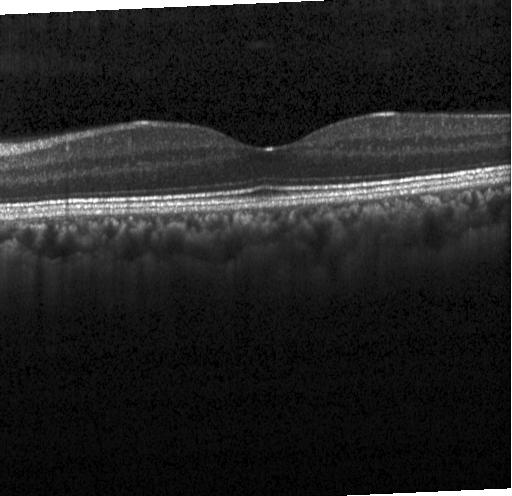
Optical coherence tomography B-scan, SD-OCT, instrument: Heidelberg Spectralis.
Macular OCT: no CNV, DME, or drusen.